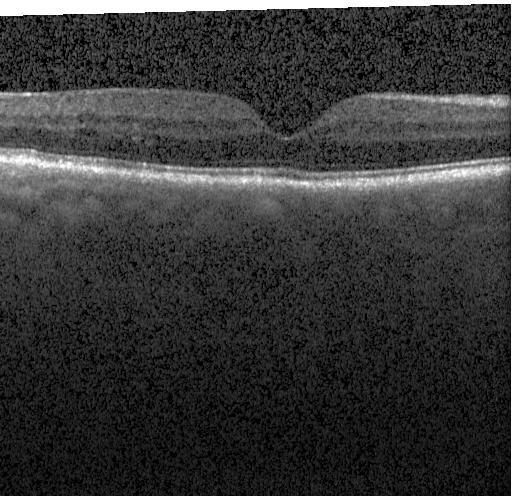

Optical coherence tomography scan. Instrument: Heidelberg Spectralis — This B-scan demonstrates no CNV, DME, or drusen.